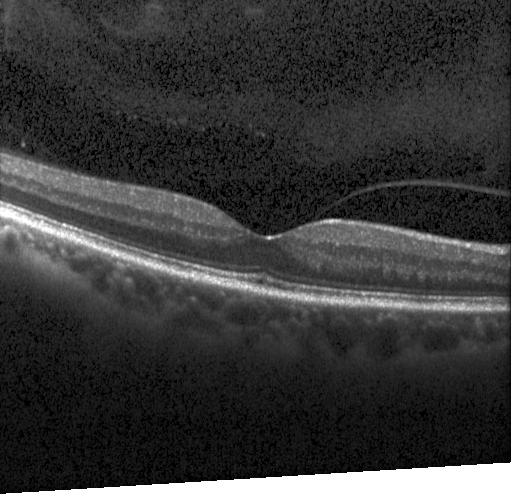

Retinal OCT cross-section showing neither choroidal neovascularization, diabetic macular edema, nor drusen.